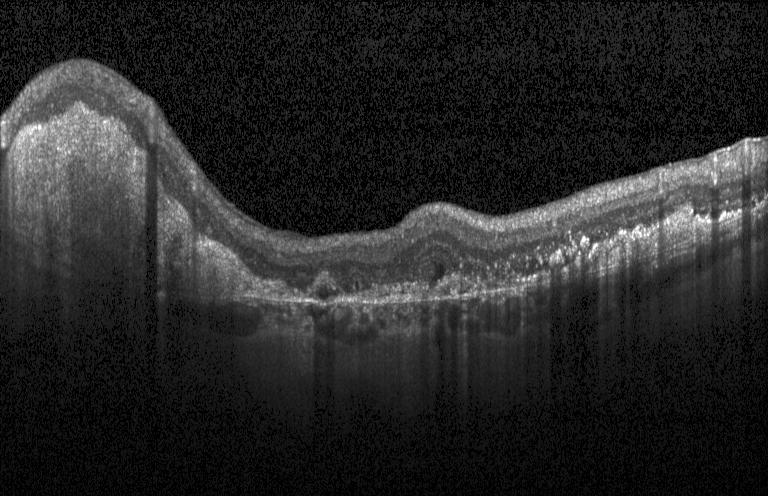 Heidelberg Spectralis. Retinal OCT B-scan — Assessment: a choroidal neovascular membrane.